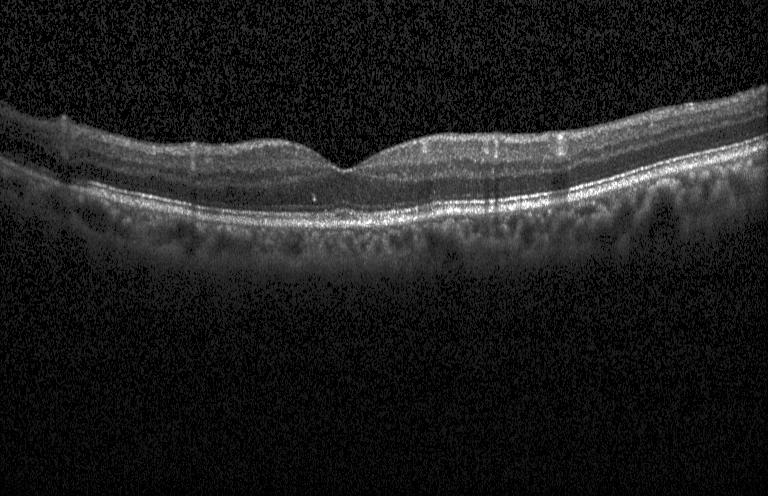 Heidelberg Spectralis OCT system; OCT line scan. Finding: no CNV, DME, or drusen.